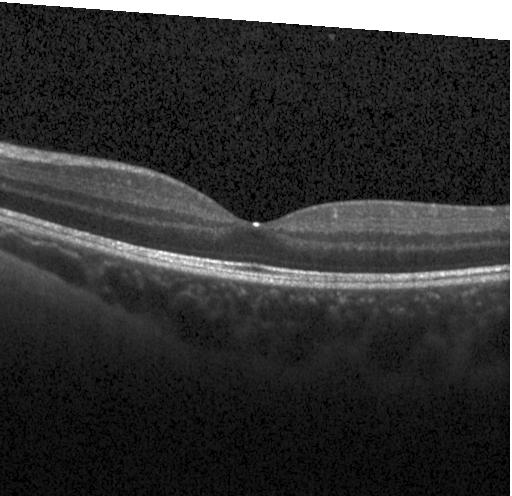
Retinal OCT B-scan.
Impression: neither choroidal neovascularization, diabetic macular edema, nor drusen.